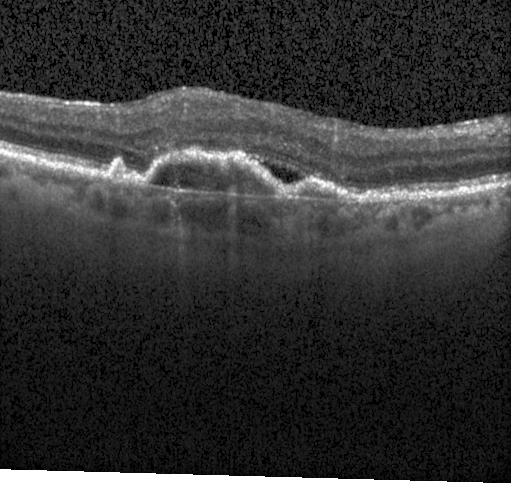

OCT line scan
Macular OCT: choroidal neovascularization (CNV).